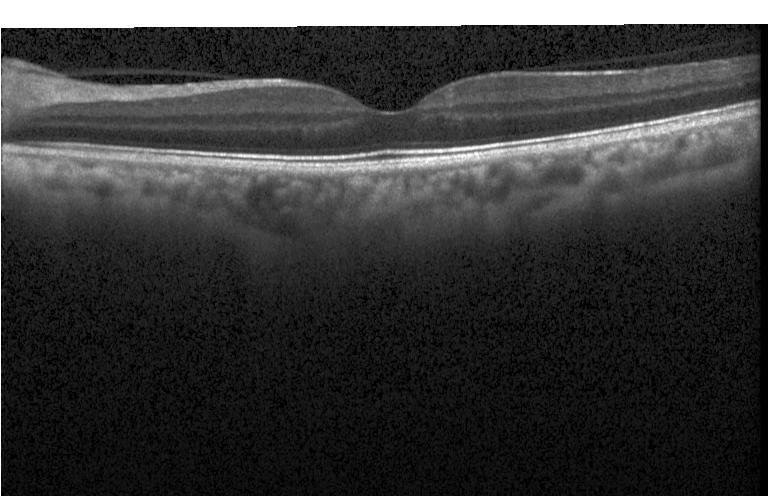
Diagnosis: no evidence of CNV, DME, or drusen.